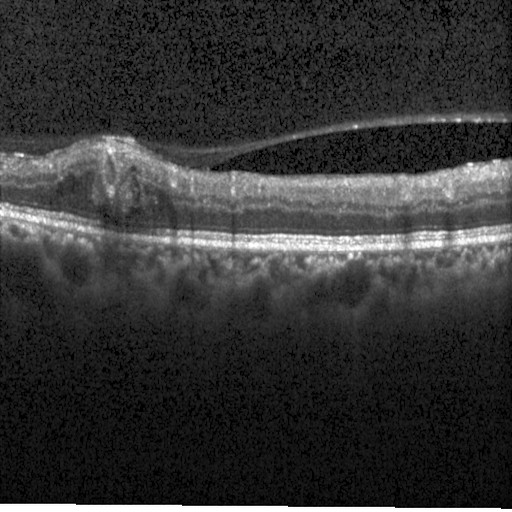

OCT line scan · macular scan · acquired on a Heidelberg Spectralis · spectral-domain OCT. Diagnosis: diabetic macular edema.